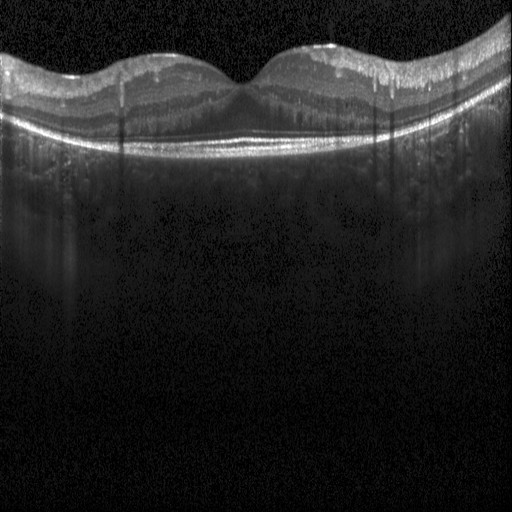 Retinal OCT cross-section showing diabetic macular edema.